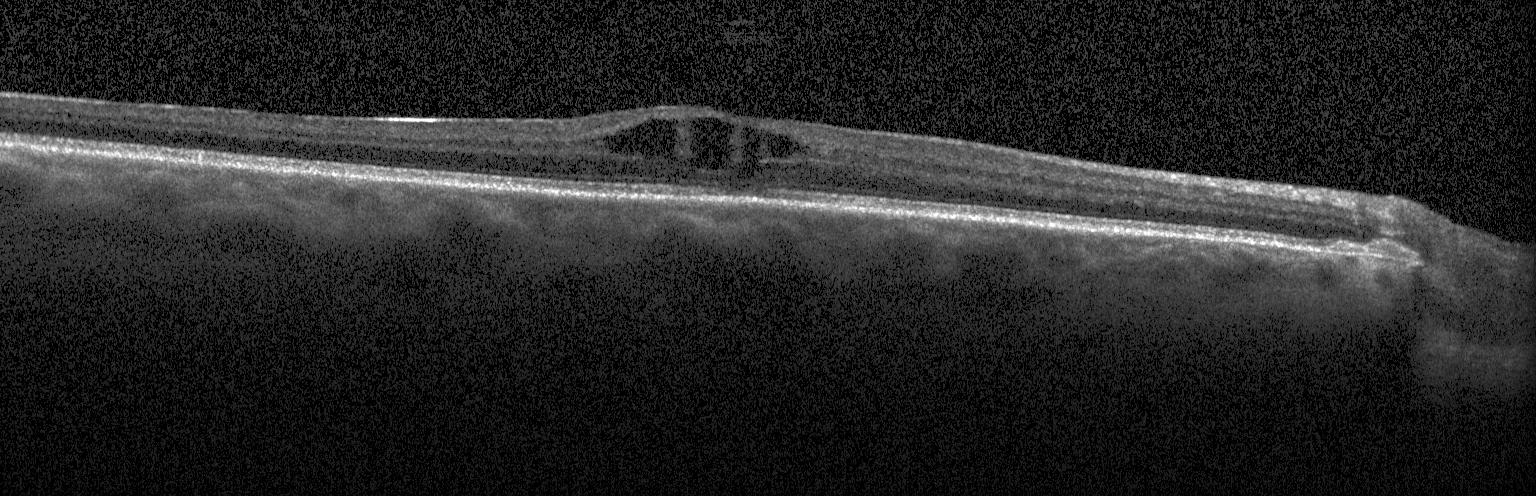

Impression: diabetic macular edema (DME).